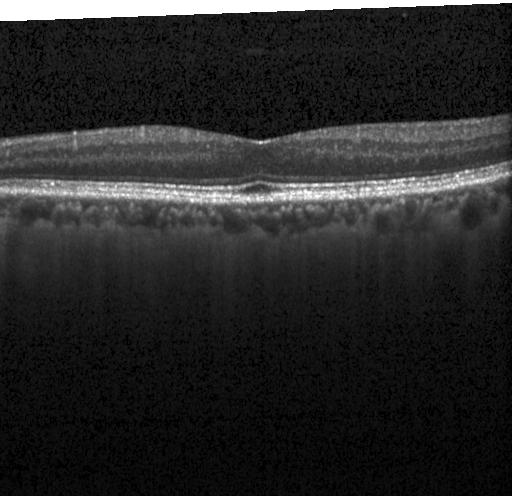 OCT B-scan; centered on the fovea; acquired on a Heidelberg Spectralis — Diagnosis: no choroidal neovascularization, diabetic macular edema, or drusen.